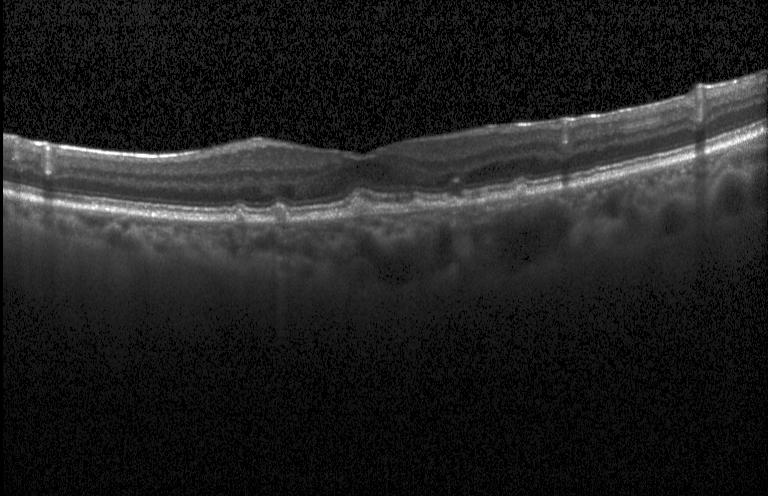 Retinal OCT B-scan
Impression: sub-RPE drusenoid deposits.